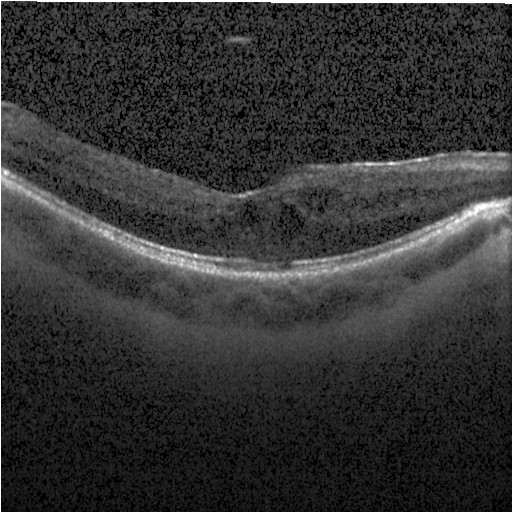 Heidelberg Spectralis OCT system · OCT B-scan — This B-scan demonstrates DME.